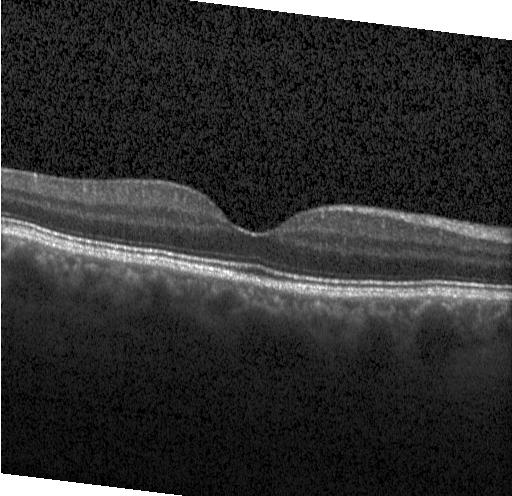 Spectral-domain optical coherence tomography. Retinal OCT B-scan. Centered on the fovea. Macular OCT: no CNV, no DME, and no drusen.